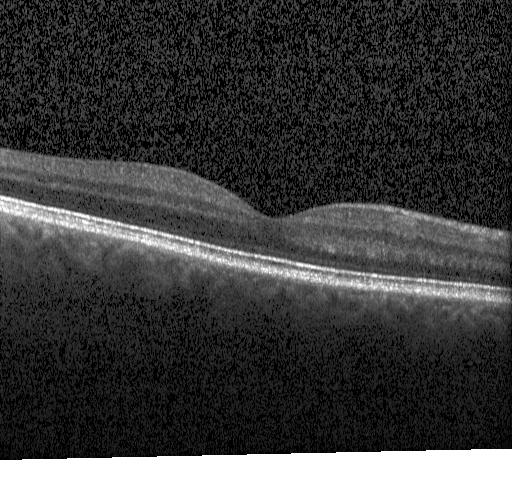
Heidelberg Spectralis OCT system; centered on the fovea; OCT B-scan — Assessment: no choroidal neovascularization, diabetic macular edema, or drusen.